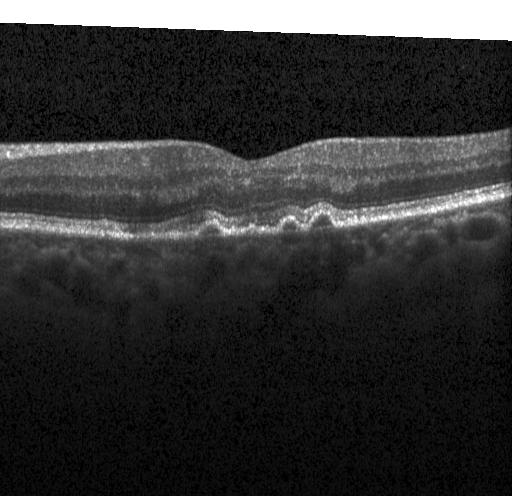
Retinal OCT cross-section; SD-OCT.
Finding: sub-RPE drusenoid deposits.